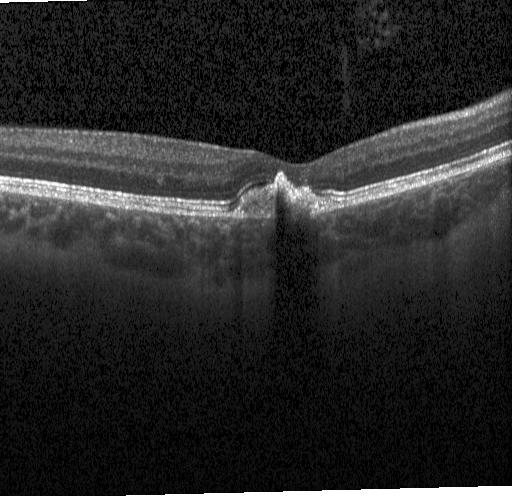

Macular scan, spectral-domain optical coherence tomography, Heidelberg Spectralis OCT system, optical coherence tomography scan.
Macular OCT: choroidal neovascularization.